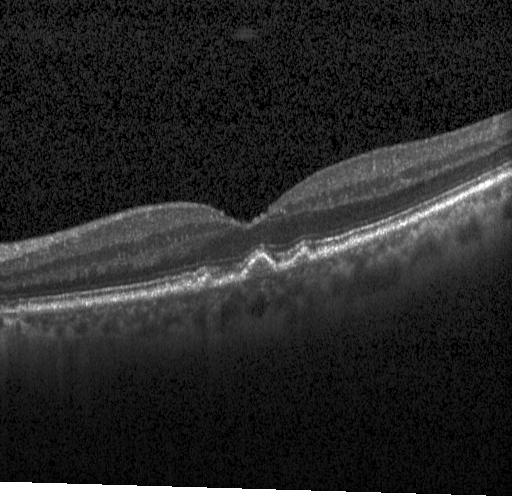
Retinal OCT cross-section showing multiple drusen.